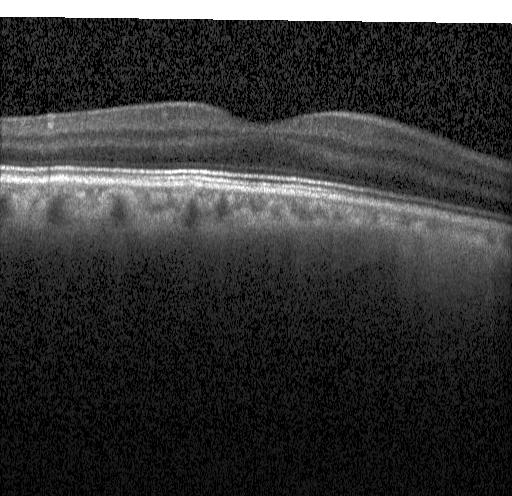 Spectral-domain optical coherence tomography. Optical coherence tomography scan. Through the macula.
Impression: no CNV, DME, or drusen.